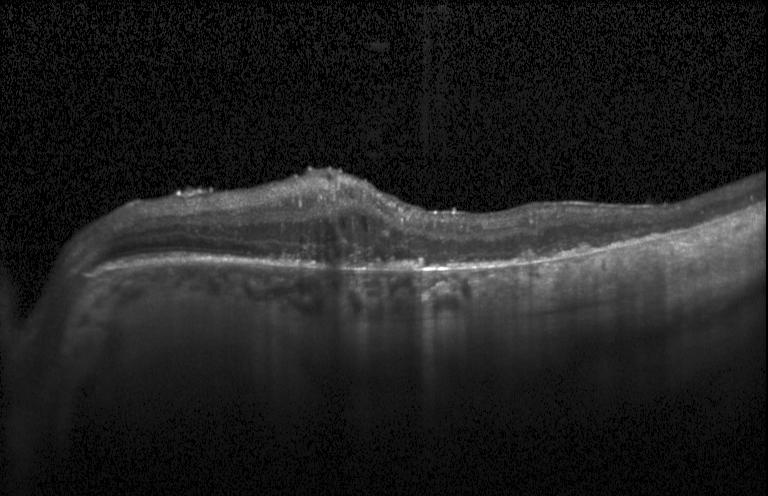

Optical coherence tomography B-scan
Macular OCT: DME.